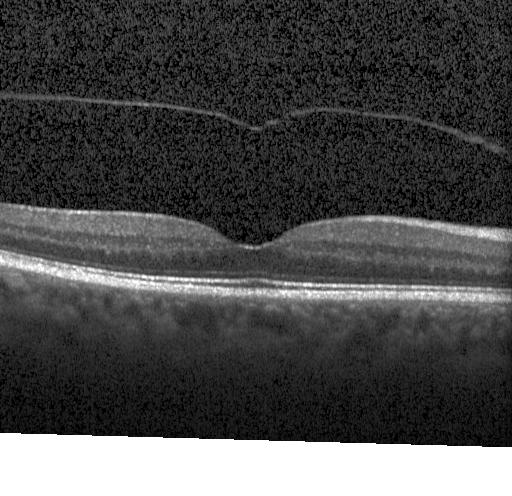

Retinal OCT cross-section showing no evidence of CNV, DME, or drusen.